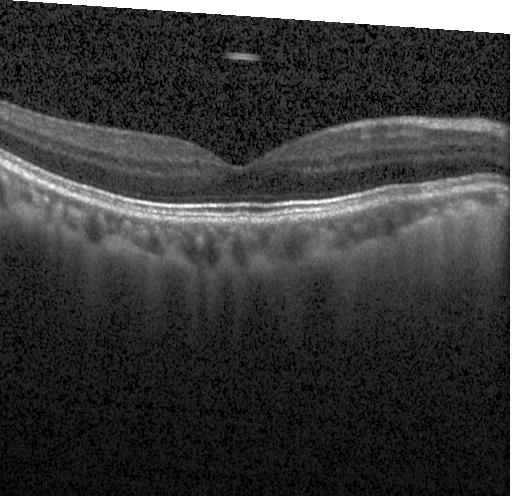
Macular scan · optical coherence tomography scan. Diagnosis: no evidence of CNV, DME, or drusen.